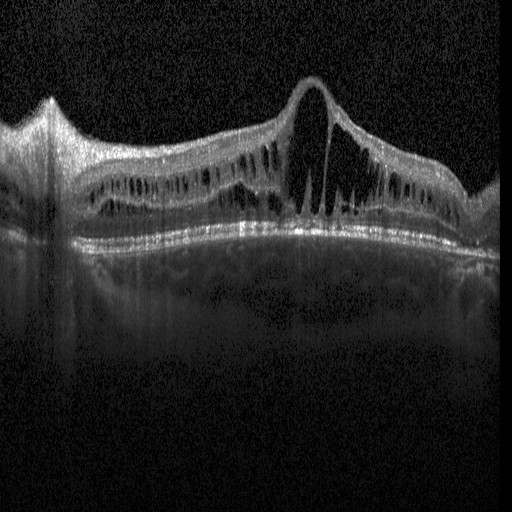
Macular OCT: DME.